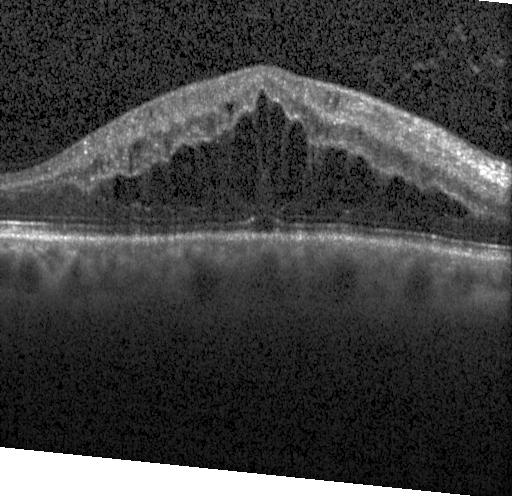
Through the macula, instrument: Heidelberg Spectralis, OCT B-scan
Finding: DME.